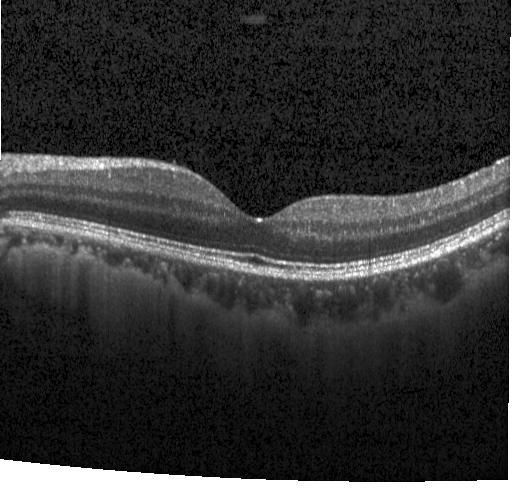 Finding: no choroidal neovascularization, diabetic macular edema, or drusen.